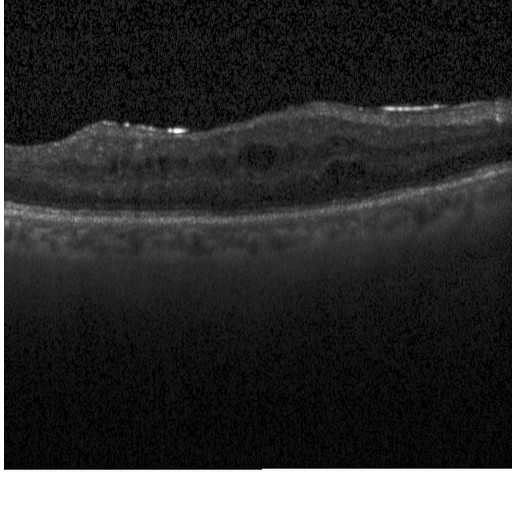 Spectral-domain optical coherence tomography · fovea-centered · Heidelberg Spectralis · optical coherence tomography scan.
Finding: diabetic macular edema (DME).